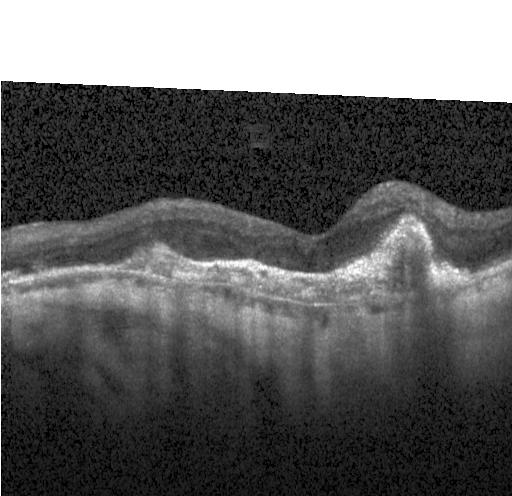
OCT line scan, Heidelberg Spectralis OCT system, spectral-domain optical coherence tomography, fovea-centered. Impression: choroidal neovascularization.